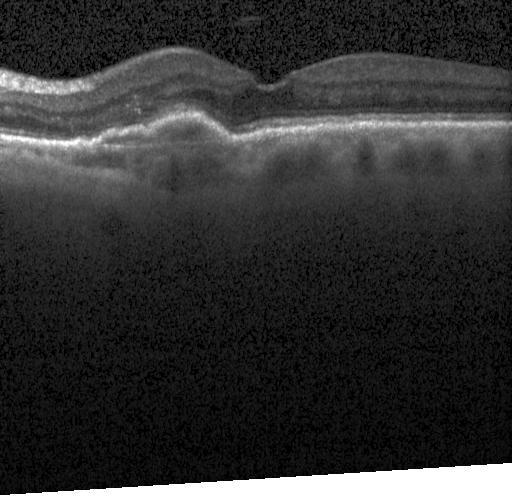 This B-scan demonstrates CNV.